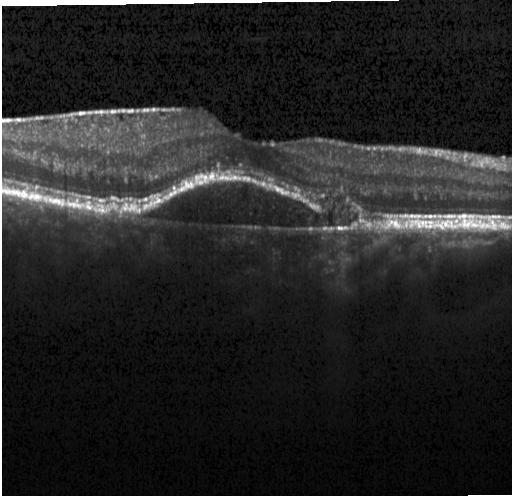

Macular OCT: choroidal neovascularization (CNV).